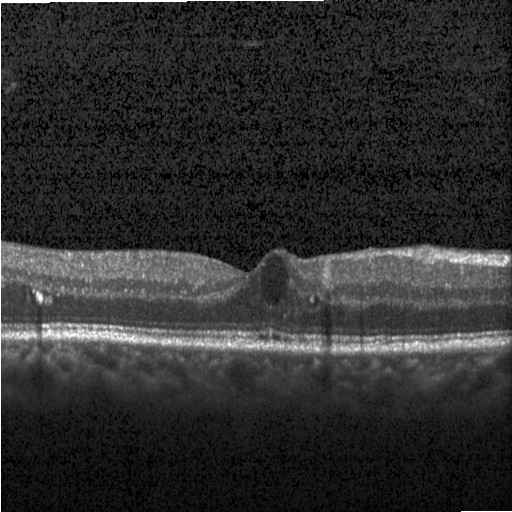 OCT B-scan. Centered on the fovea. SD-OCT. Acquired on a Heidelberg Spectralis.
Impression: DME.